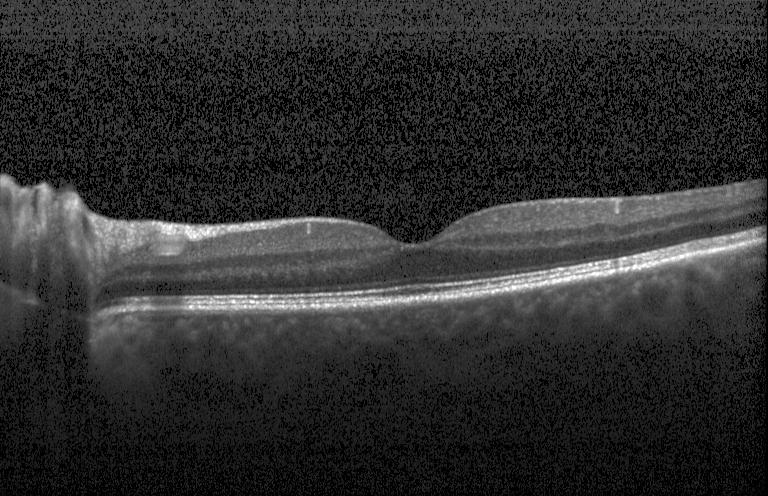 Impression: neither choroidal neovascularization, diabetic macular edema, nor drusen.